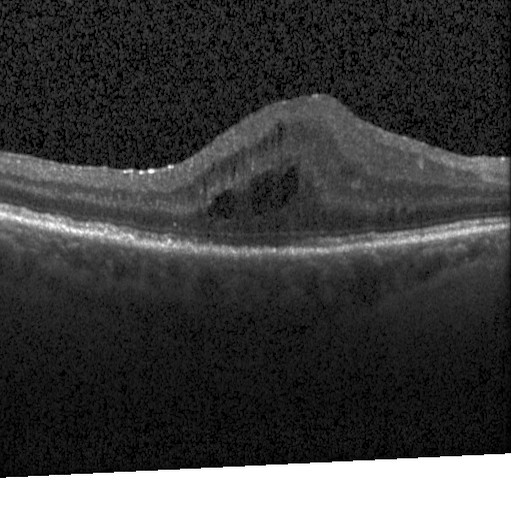 Macular OCT: diabetic macular edema (DME).